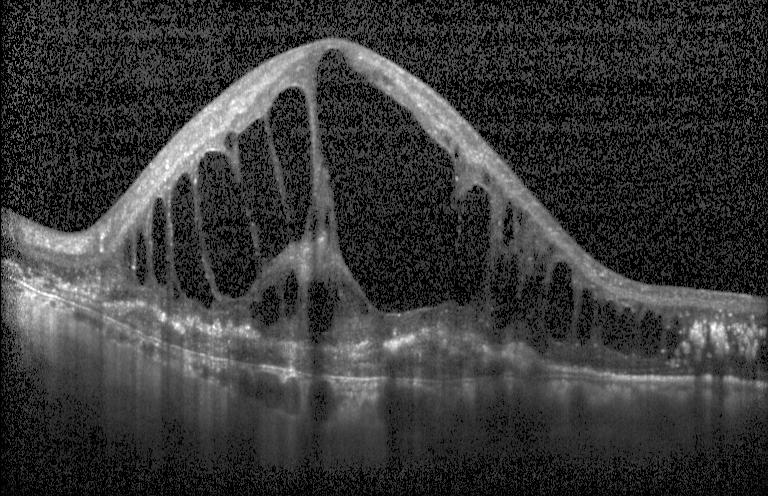

Spectral-domain OCT B-scan: choroidal neovascularization.